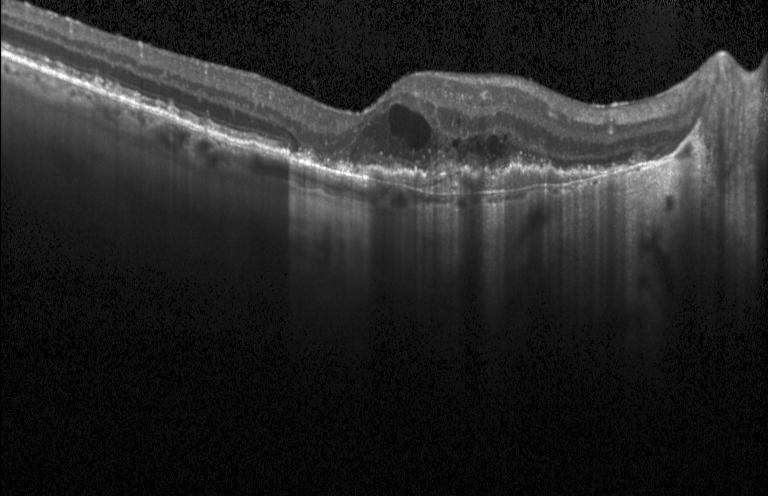

OCT B-scan — Finding: a choroidal neovascular membrane.